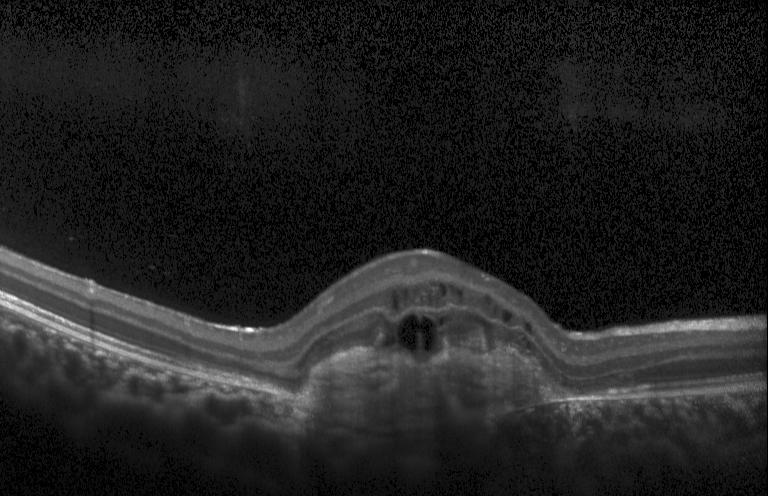 OCT scan showing a choroidal neovascular membrane.